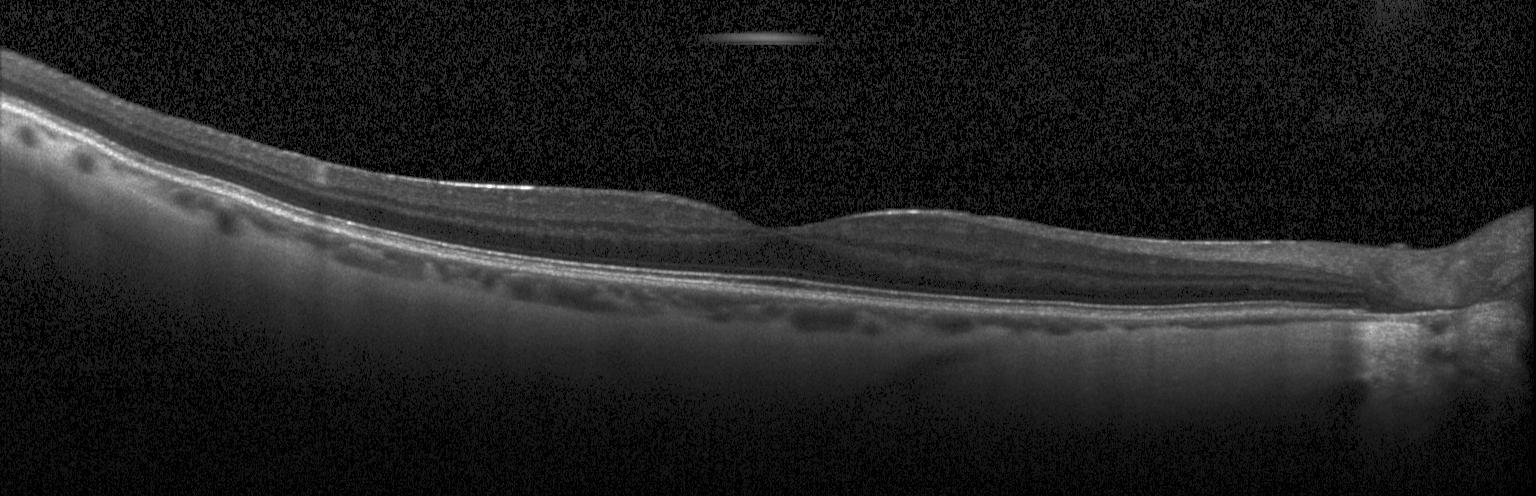 Spectral-domain OCT B-scan: no choroidal neovascularization, no diabetic macular edema, and no drusen.